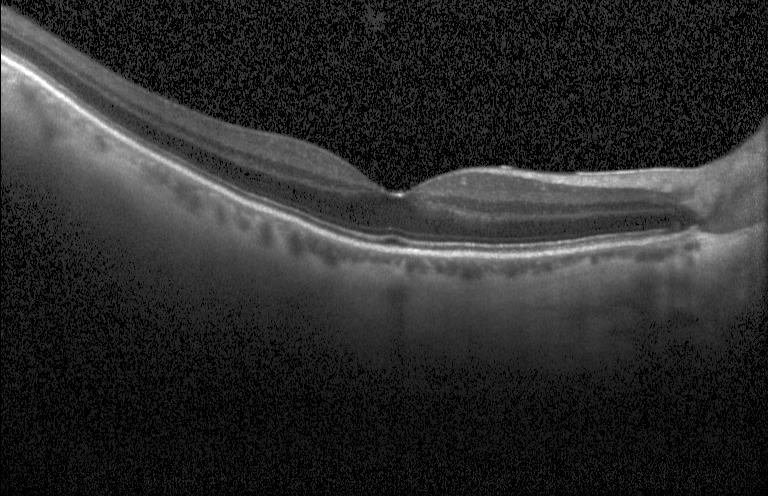

Retinal OCT cross-section.
Assessment: no CNV, DME, or drusen.